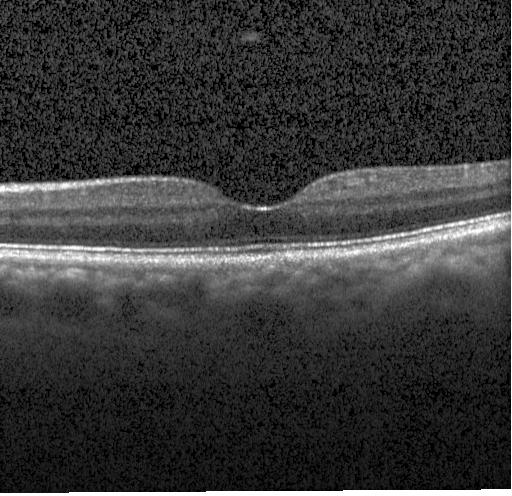
Centered on the fovea · OCT line scan · instrument: Heidelberg Spectralis.
Impression: no choroidal neovascularization, no diabetic macular edema, and no drusen.